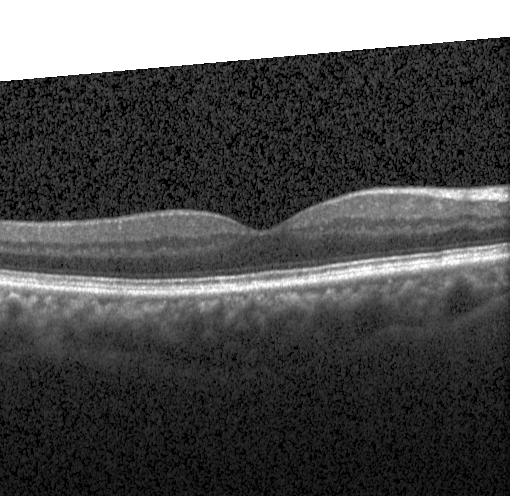 Heidelberg Spectralis; optical coherence tomography B-scan; spectral-domain optical coherence tomography; through the macula. Assessment: no evidence of CNV, DME, or drusen.